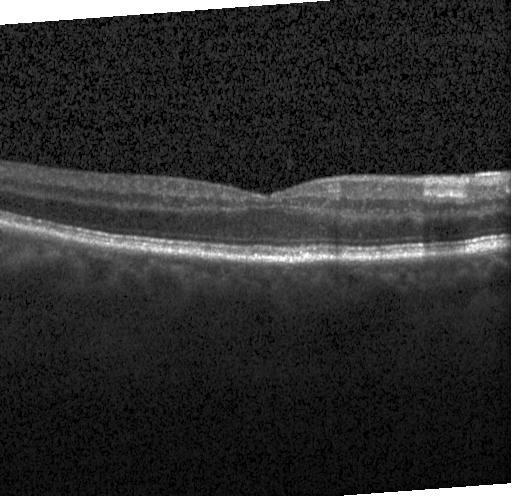 Diagnosis: no CNV, no DME, and no drusen.